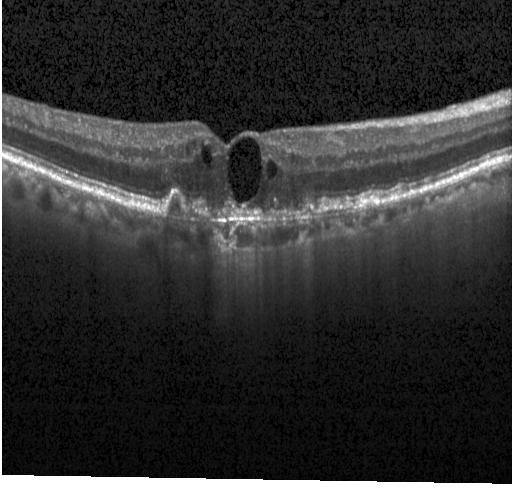

Macular scan. Optical coherence tomography B-scan. Spectral-domain optical coherence tomography. Heidelberg Spectralis OCT system
The scan shows a choroidal neovascular membrane.